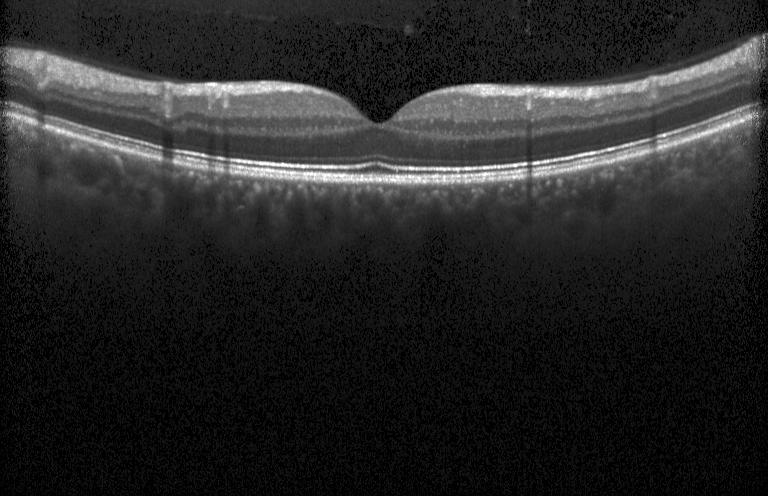 Optical coherence tomography scan · instrument: Heidelberg Spectralis · spectral-domain OCT.
Assessment: no evidence of choroidal neovascularization, diabetic macular edema, or drusen.